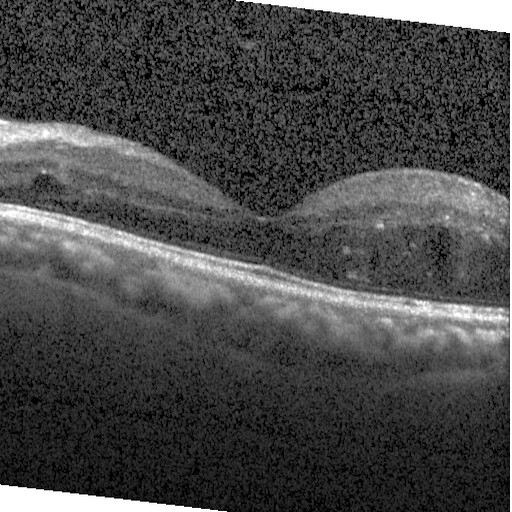

OCT B-scan — This B-scan demonstrates diabetic macular edema.